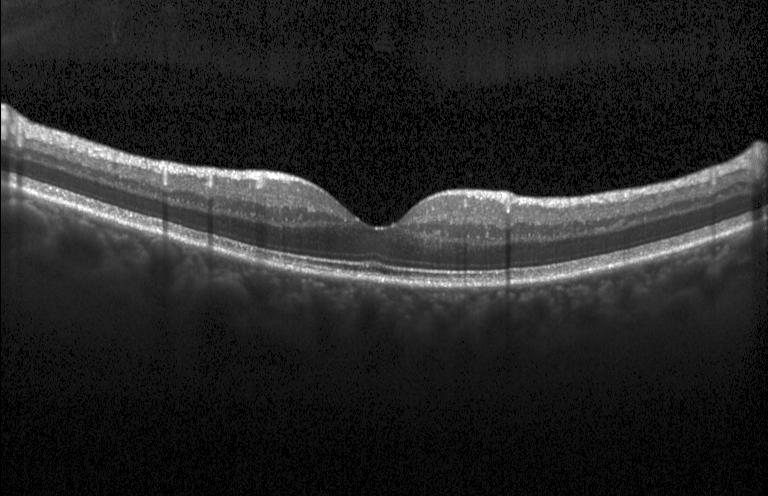

OCT B-scan showing neither choroidal neovascularization, diabetic macular edema, nor drusen.